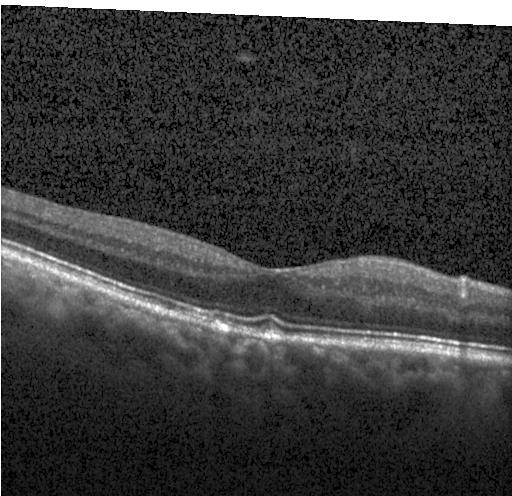
Diagnosis: sub-RPE drusenoid deposits.